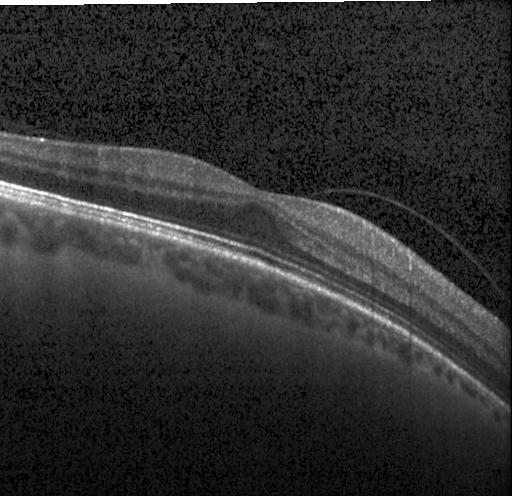

Horizontal scan through the fovea · OCT B-scan.
Impression: no choroidal neovascularization, no diabetic macular edema, and no drusen.